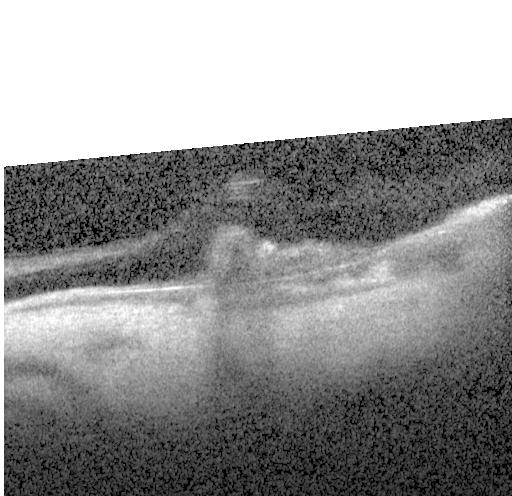 OCT finding: choroidal neovascularization.